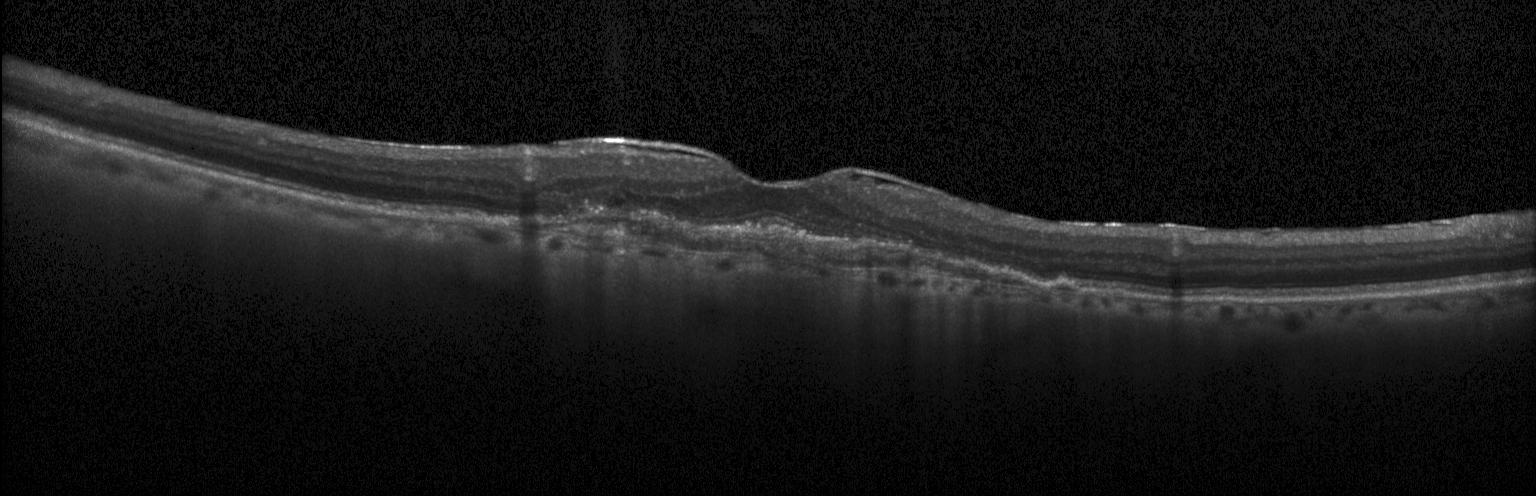

OCT B-scan showing choroidal neovascularization.